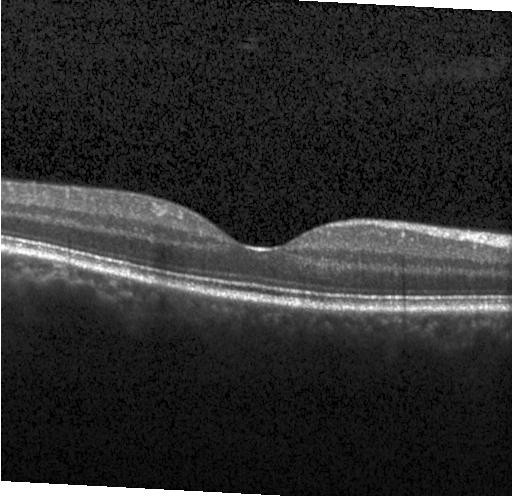
This B-scan demonstrates no CNV, DME, or drusen.